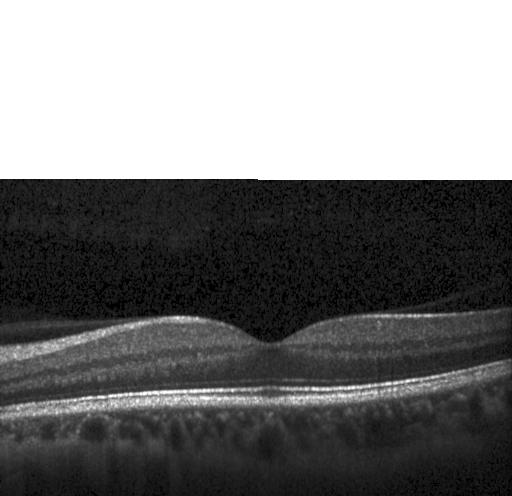

Optical coherence tomography scan. Spectral-domain OCT. Centered on the fovea. Acquired on a Heidelberg Spectralis. Diagnosis: no choroidal neovascularization, diabetic macular edema, or drusen.